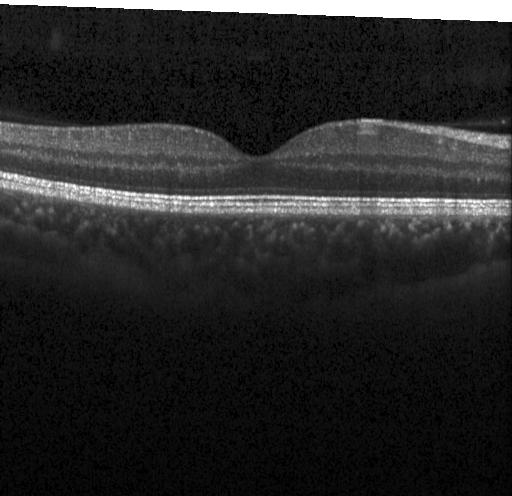

OCT B-scan
OCT finding: neither CNV, DME, nor drusen.